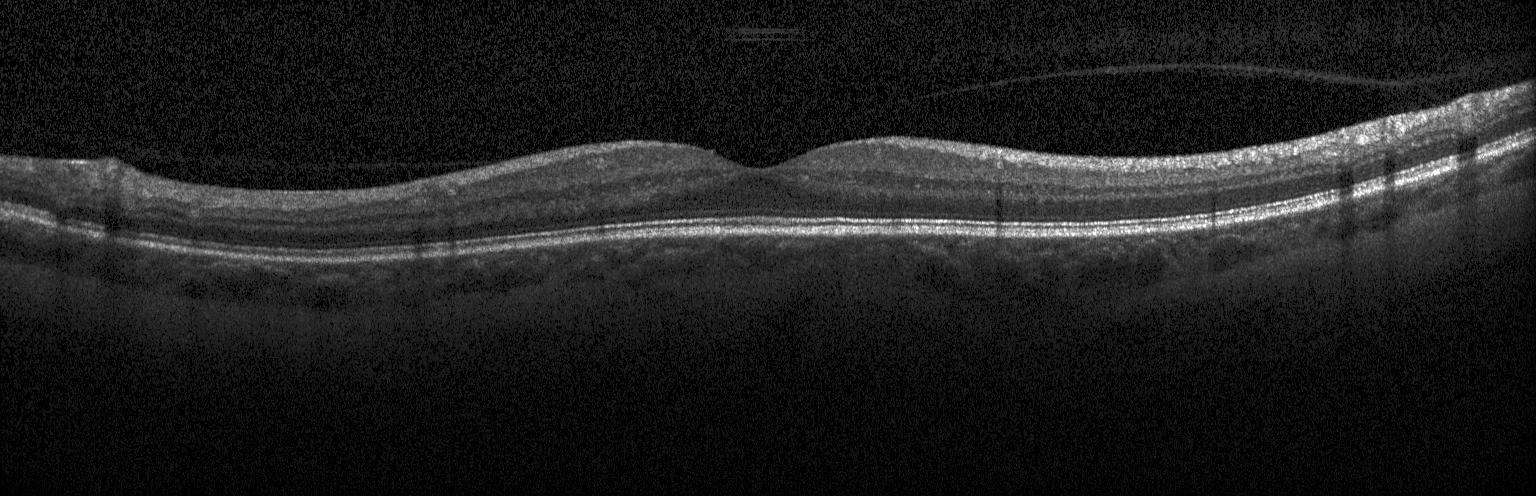
OCT B-scan, centered on the fovea, SD-OCT — Macular OCT: no evidence of choroidal neovascularization, diabetic macular edema, or drusen.